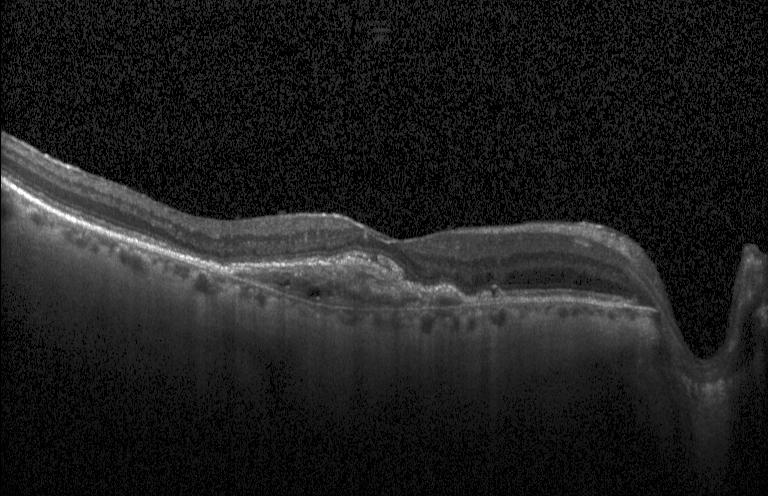 Optical coherence tomography B-scan.
Impression: CNV.